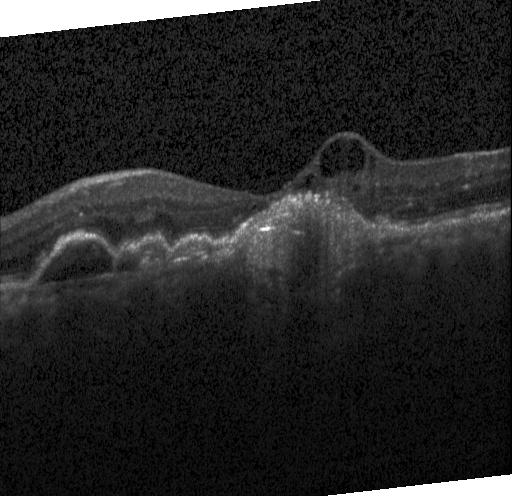
Optical coherence tomography B-scan · horizontal scan through the fovea · spectral-domain optical coherence tomography · Heidelberg Spectralis.
This B-scan demonstrates choroidal neovascularization (CNV).